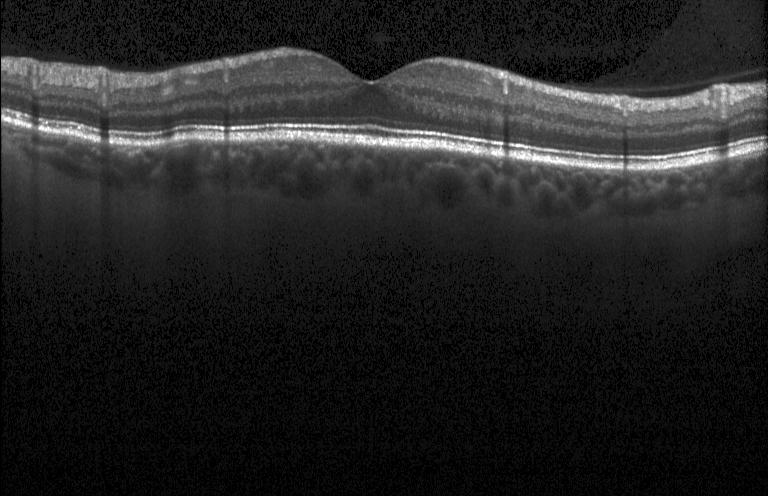

OCT B-scan · fovea-centered · SD-OCT · instrument: Heidelberg Spectralis. No choroidal neovascularization, no diabetic macular edema, and no drusen.